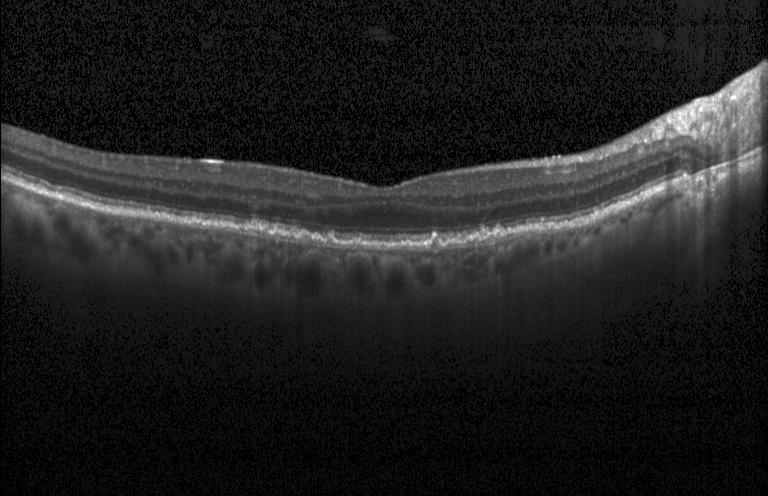

Optical coherence tomography B-scan. SD-OCT
Finding: multiple drusen.